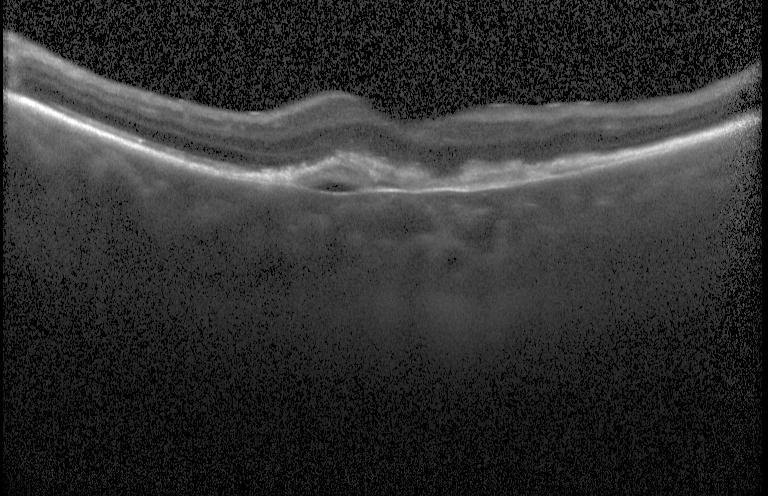 Optical coherence tomography scan · SD-OCT · centered on the fovea · instrument: Heidelberg Spectralis — Assessment: a choroidal neovascular membrane.